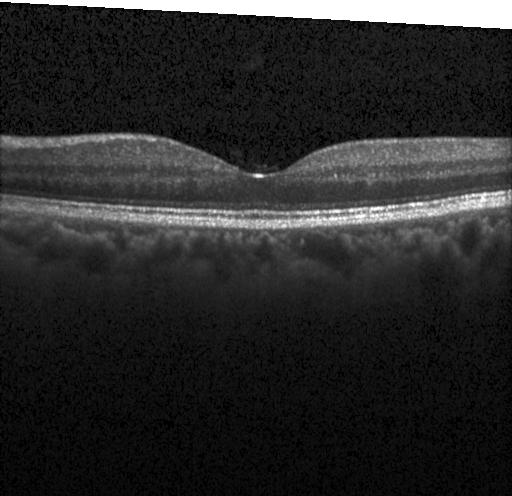 Spectral-domain OCT, Heidelberg Spectralis OCT system, OCT line scan, fovea-centered. Impression: neither choroidal neovascularization, diabetic macular edema, nor drusen.